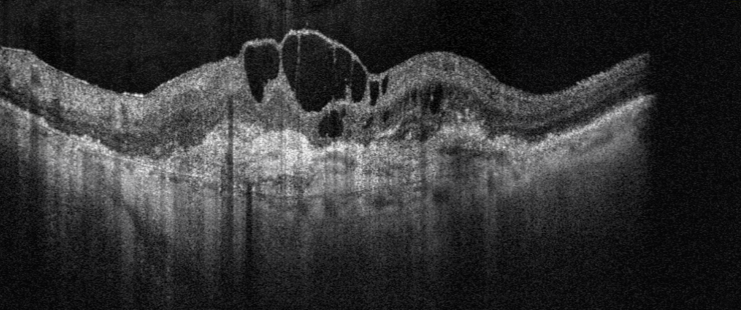
OCT B-scan · acquired on an Optovue Avanti RTVue XR · macular scan. OCT finding: AMD.